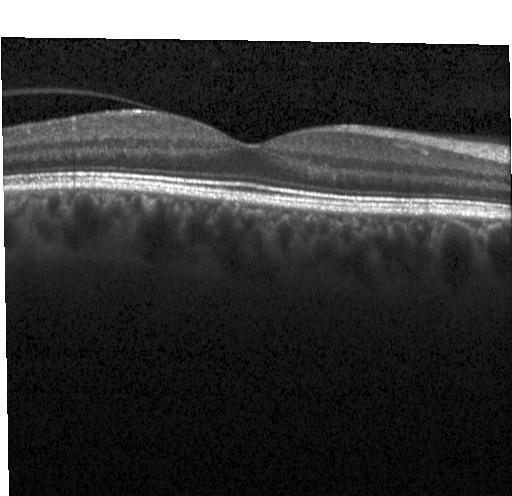 Impression: no evidence of CNV, DME, or drusen.